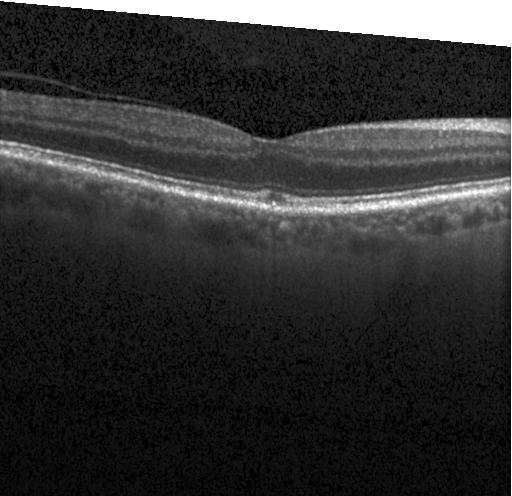 This B-scan demonstrates no choroidal neovascularization, diabetic macular edema, or drusen.